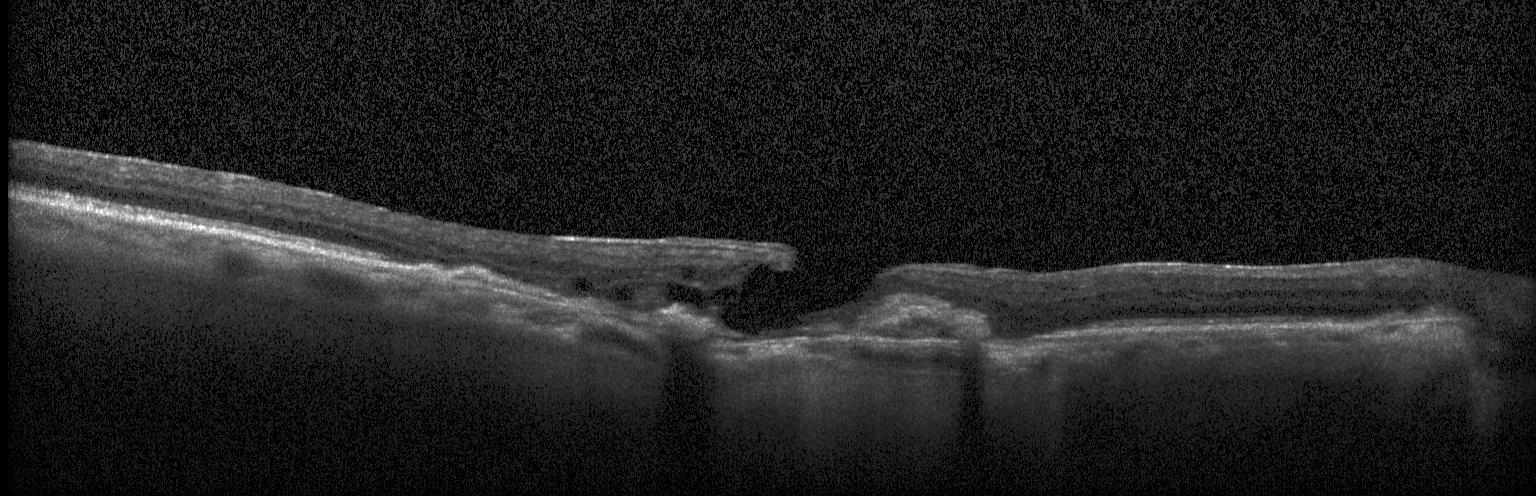 OCT B-scan — Diagnosis: choroidal neovascularization.